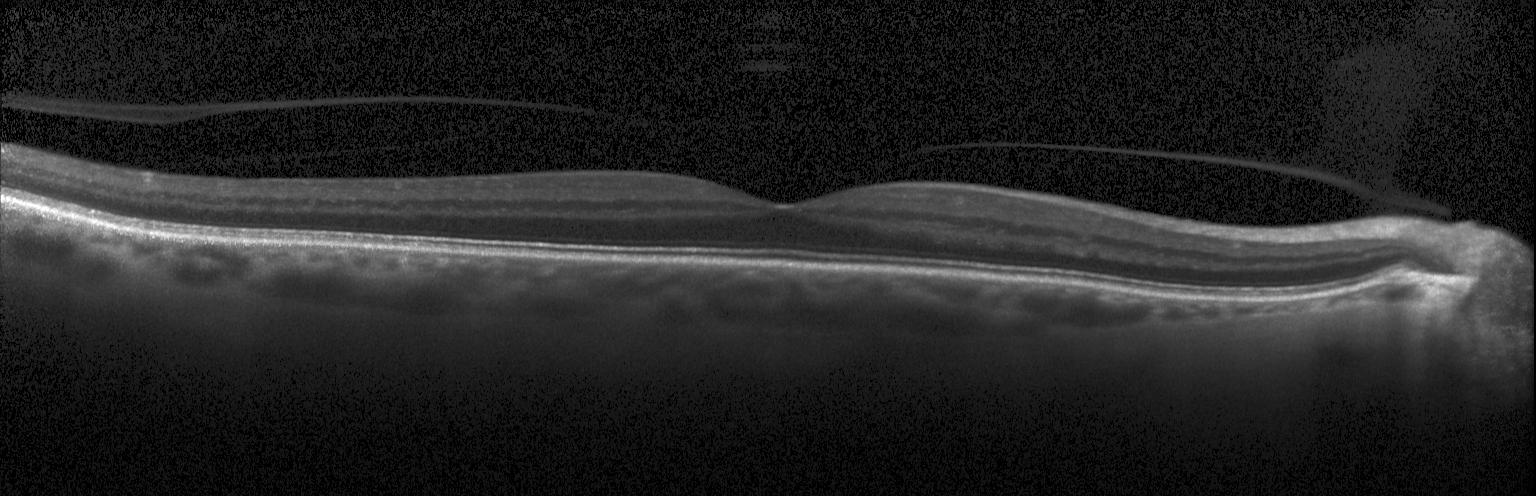
Retinal OCT B-scan, instrument: Heidelberg Spectralis, SD-OCT, fovea-centered
OCT finding: neither choroidal neovascularization, diabetic macular edema, nor drusen.